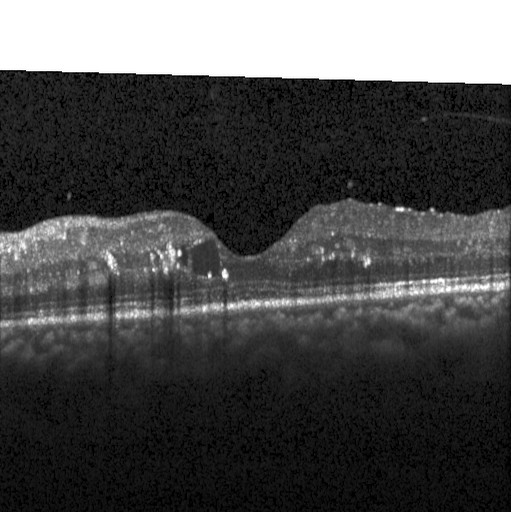
Fovea-centered · OCT line scan
Diagnosis: DME.